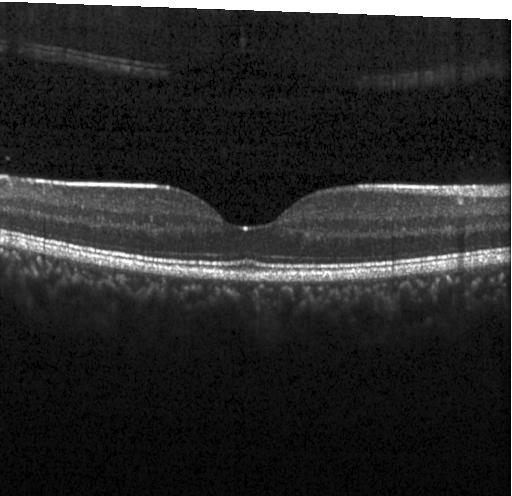
Diagnosis: no choroidal neovascularization, no diabetic macular edema, and no drusen.